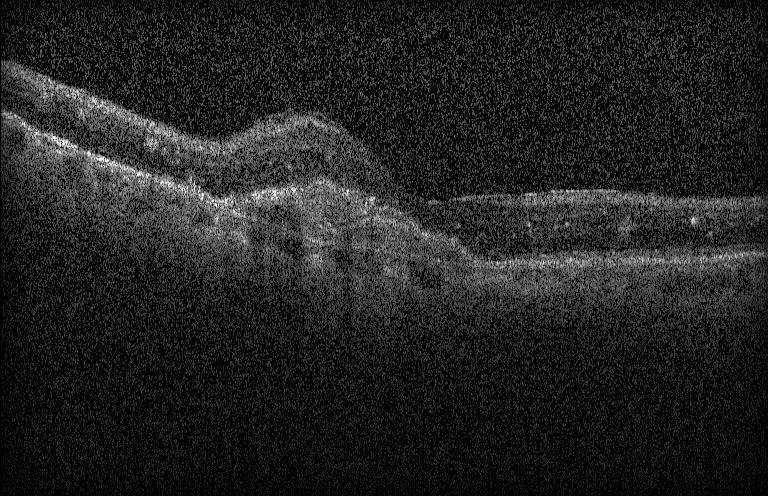

OCT line scan
Finding: a choroidal neovascular membrane.